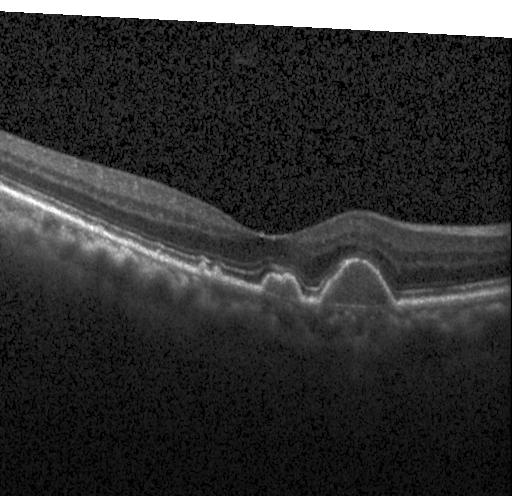 OCT B-scan showing multiple drusen.